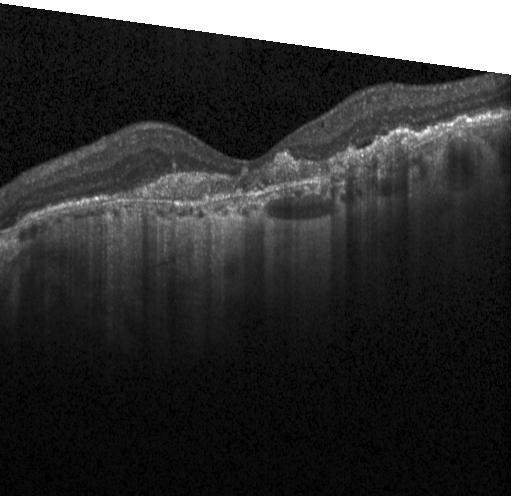

SD-OCT; OCT line scan
Diagnosis: choroidal neovascularization.